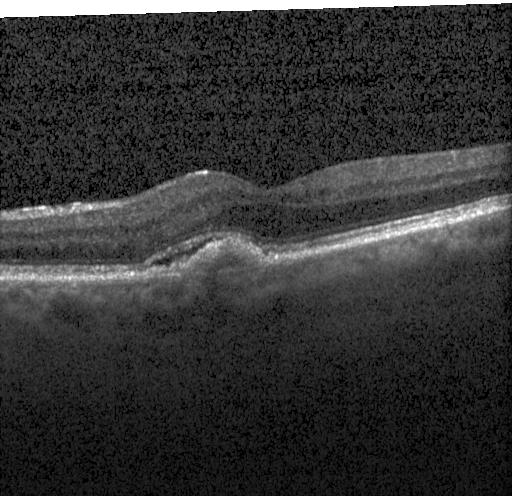
Macular OCT: a choroidal neovascular membrane.